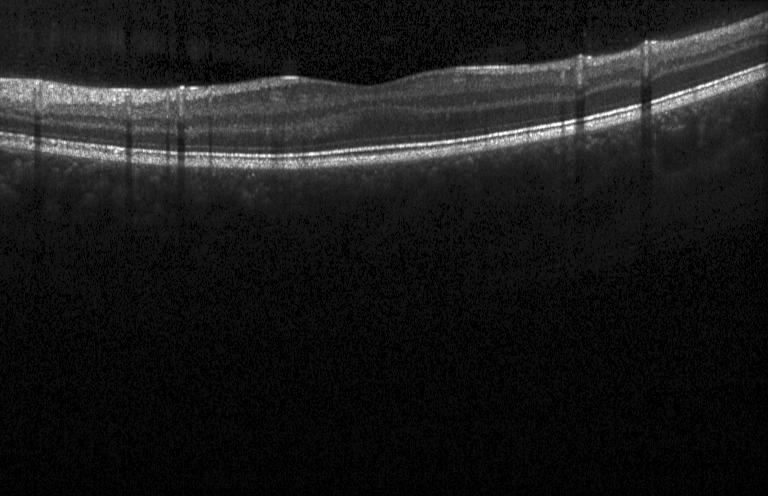

Optical coherence tomography scan. Impression: no evidence of CNV, DME, or drusen.